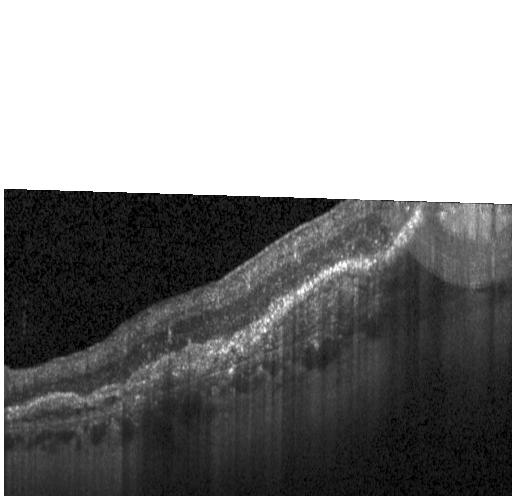

Diagnosis: CNV.